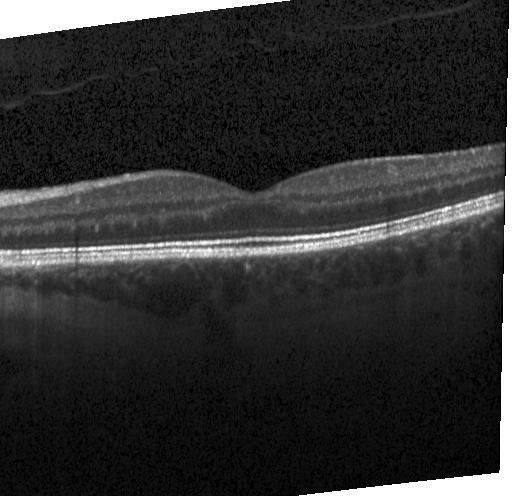

OCT finding: neither choroidal neovascularization, diabetic macular edema, nor drusen.